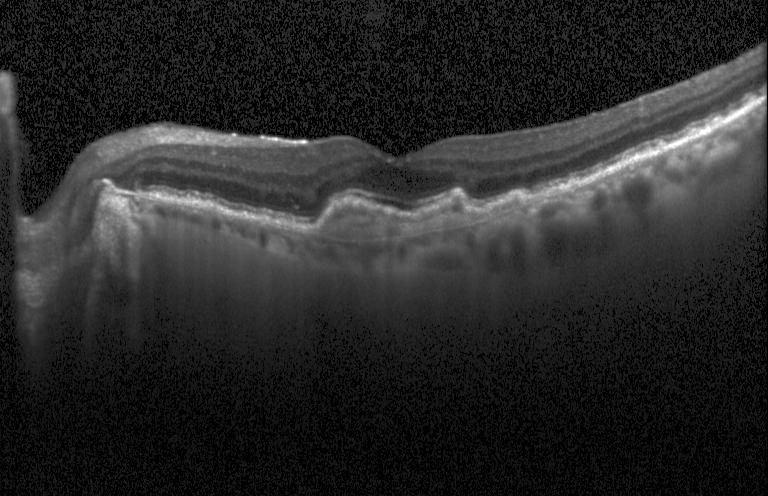

SD-OCT; horizontal scan through the fovea; retinal OCT cross-section. Assessment: a choroidal neovascular membrane.